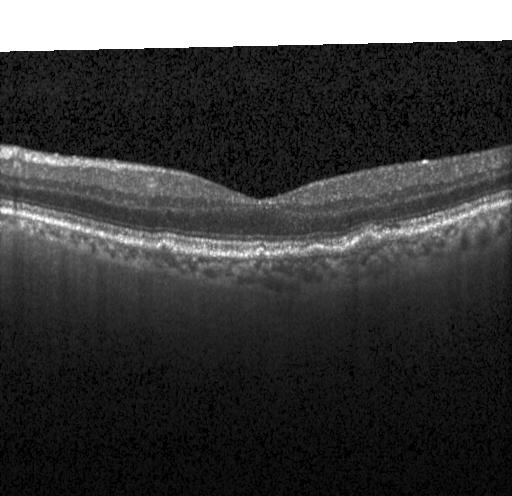 Instrument: Heidelberg Spectralis. Centered on the fovea. Spectral-domain optical coherence tomography. OCT B-scan — Finding: multiple drusen.